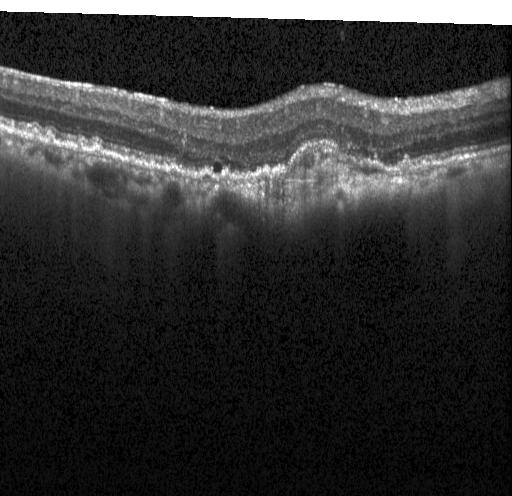 Retinal OCT B-scan. Dx: a choroidal neovascular membrane.